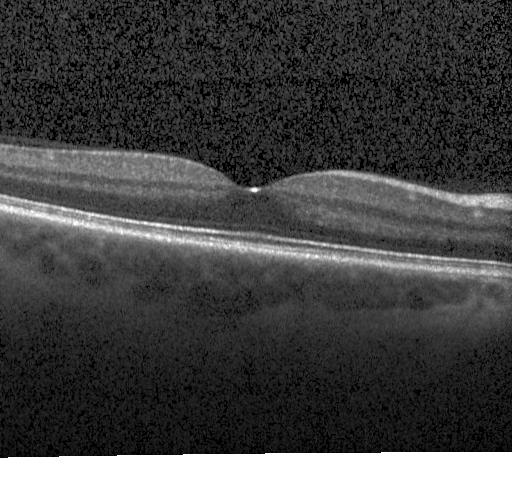
OCT line scan, Heidelberg Spectralis OCT system, through the macula. The scan shows no evidence of choroidal neovascularization, diabetic macular edema, or drusen.